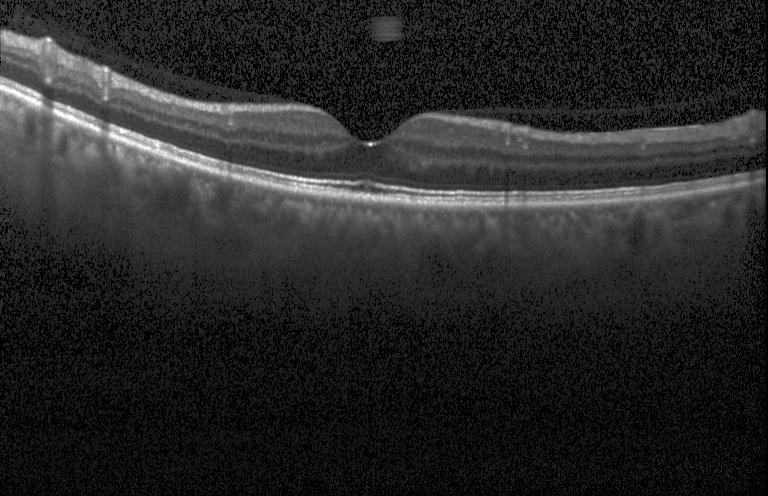
Heidelberg Spectralis · through the macula · OCT B-scan
Diagnosis: no choroidal neovascularization, no diabetic macular edema, and no drusen.